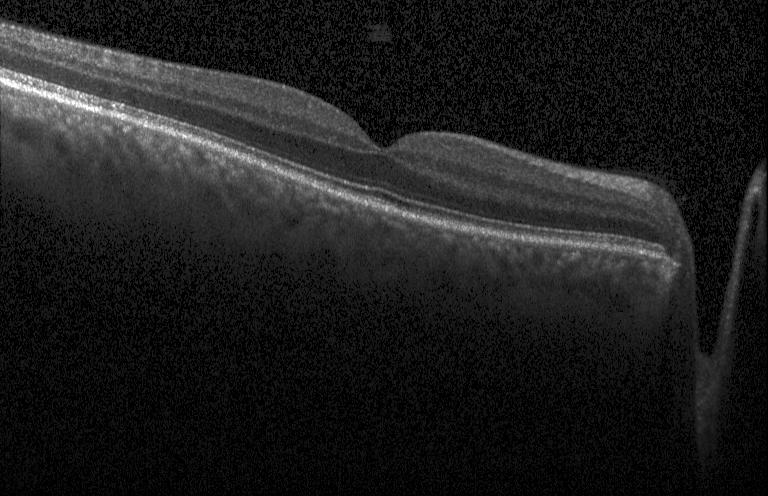

Finding: no choroidal neovascularization, diabetic macular edema, or drusen.